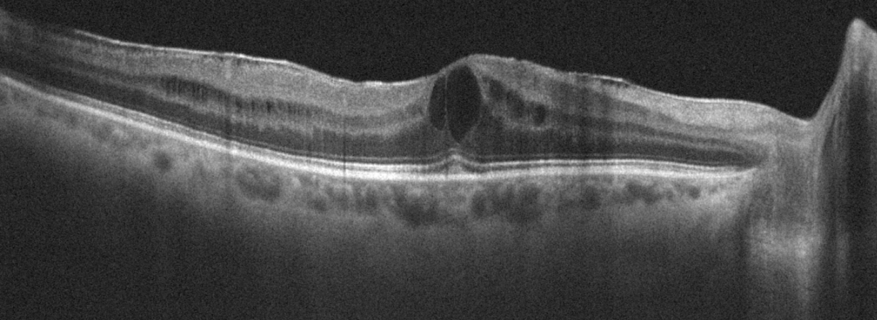 Macular OCT demonstrating diabetic macular edema (DME).